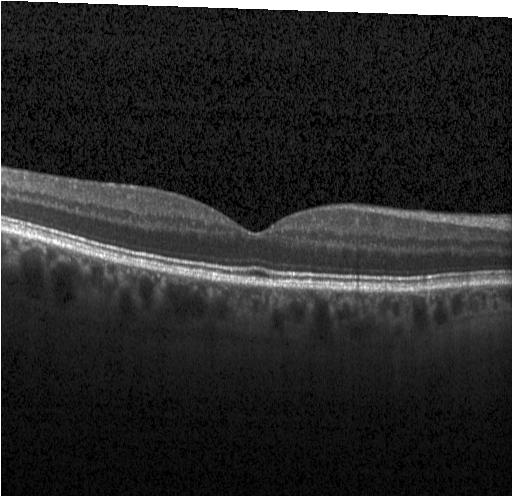 Retinal OCT cross-section
Finding: no evidence of choroidal neovascularization, diabetic macular edema, or drusen.